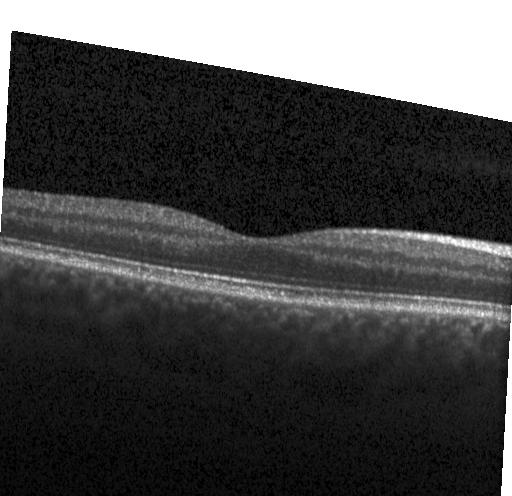

Heidelberg Spectralis · optical coherence tomography scan. This B-scan demonstrates no evidence of choroidal neovascularization, diabetic macular edema, or drusen.